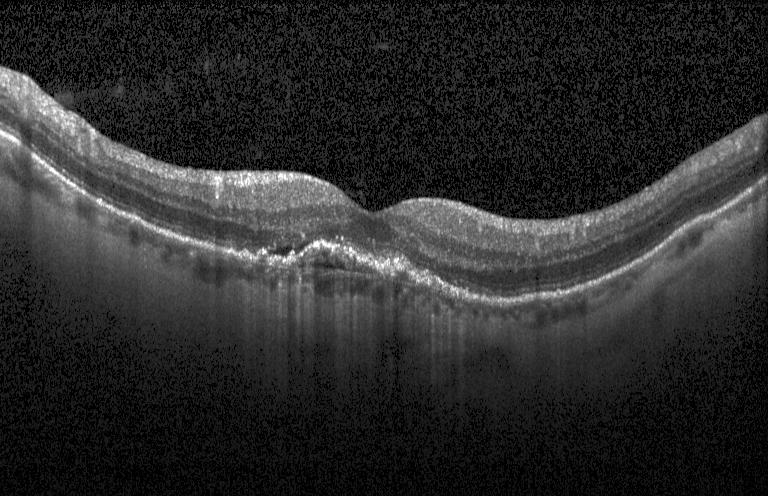
Dx: a choroidal neovascular membrane.